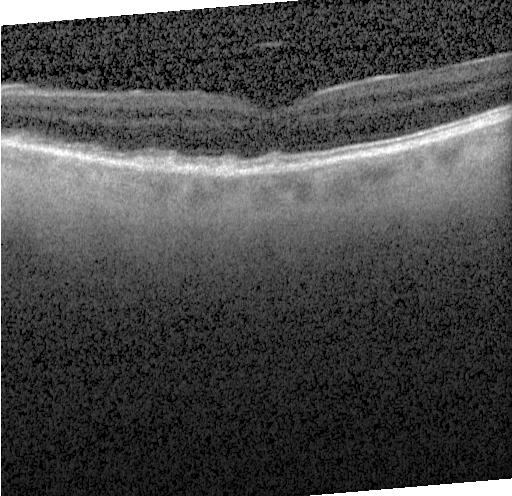
Spectral-domain OCT. Heidelberg Spectralis. Optical coherence tomography scan. Horizontal scan through the fovea — Diagnosis: drusen.